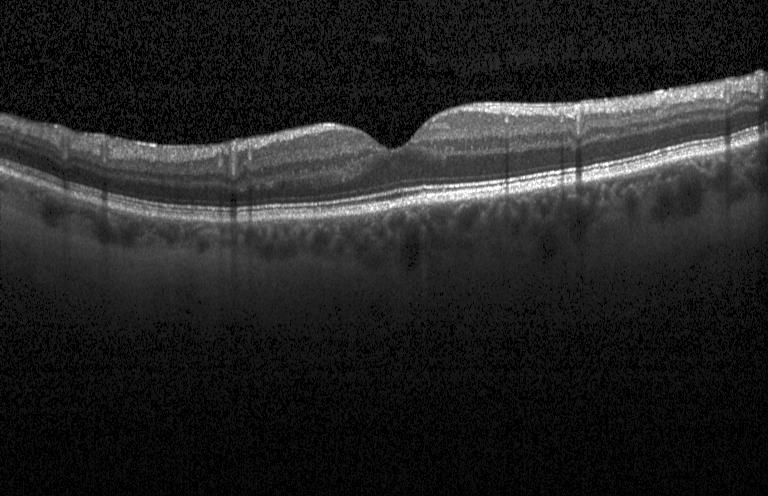 Heidelberg Spectralis. Optical coherence tomography B-scan.
The scan shows no choroidal neovascularization, no diabetic macular edema, and no drusen.